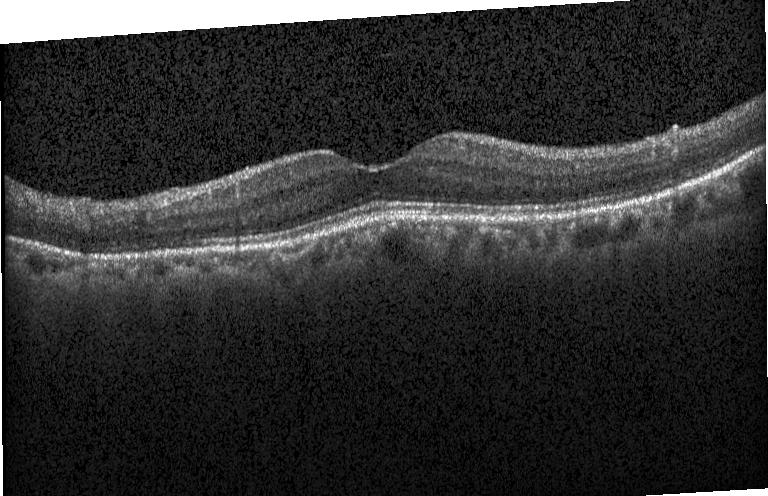

Through the macula; spectral-domain optical coherence tomography; retinal OCT B-scan — Diagnosis: no choroidal neovascularization, diabetic macular edema, or drusen.